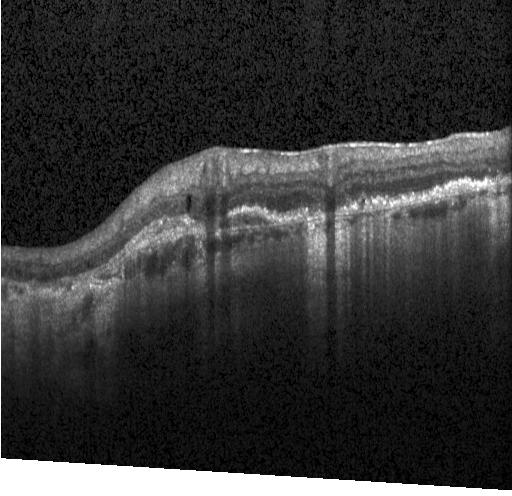

Dx: a choroidal neovascular membrane.